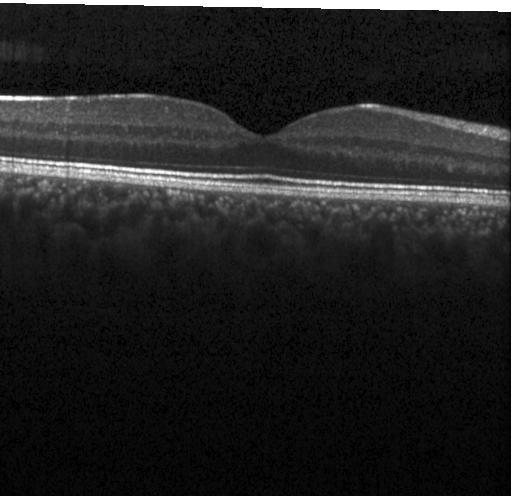 Optical coherence tomography scan · spectral-domain optical coherence tomography
Finding: neither choroidal neovascularization, diabetic macular edema, nor drusen.